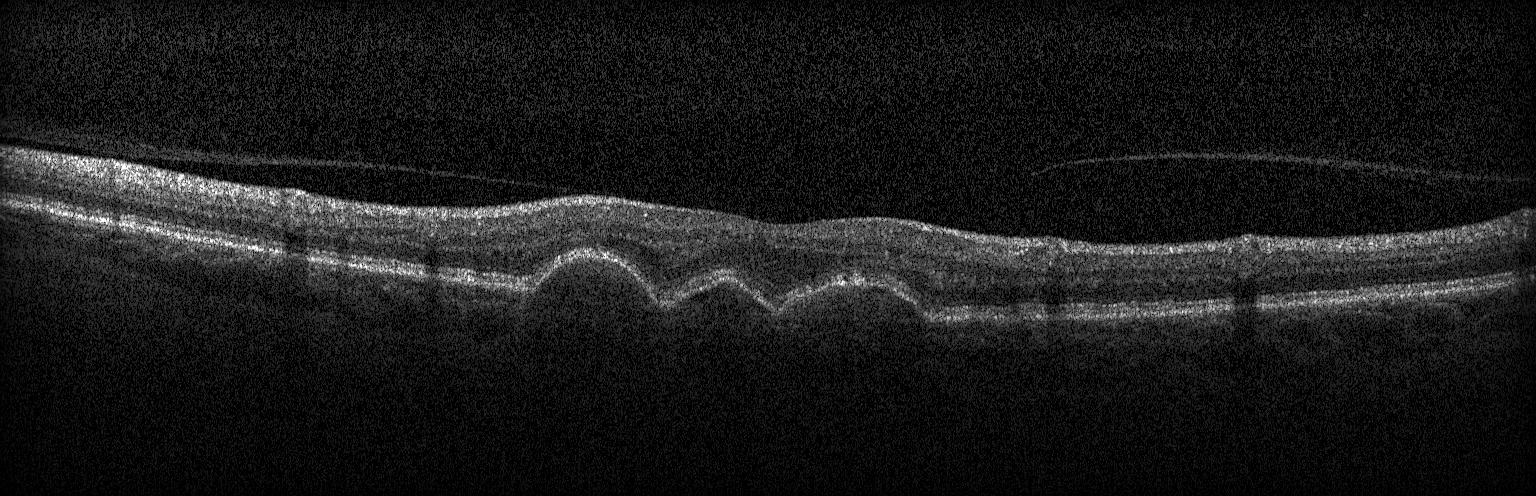
Retinal OCT B-scan. Dx: CNV.